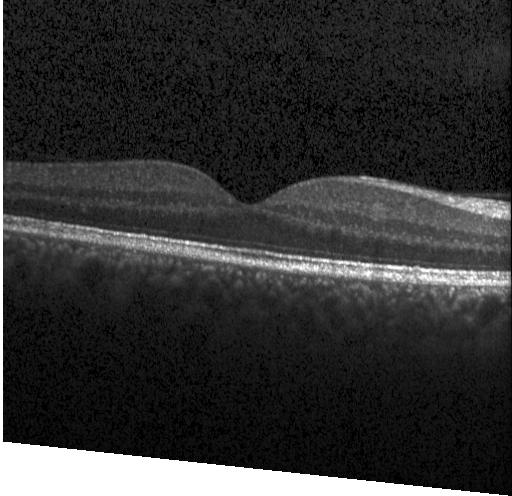
Dx: no choroidal neovascularization, diabetic macular edema, or drusen.